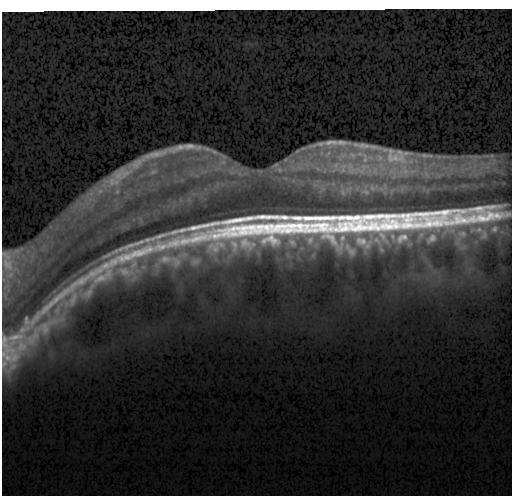

Macular OCT: no CNV, DME, or drusen.